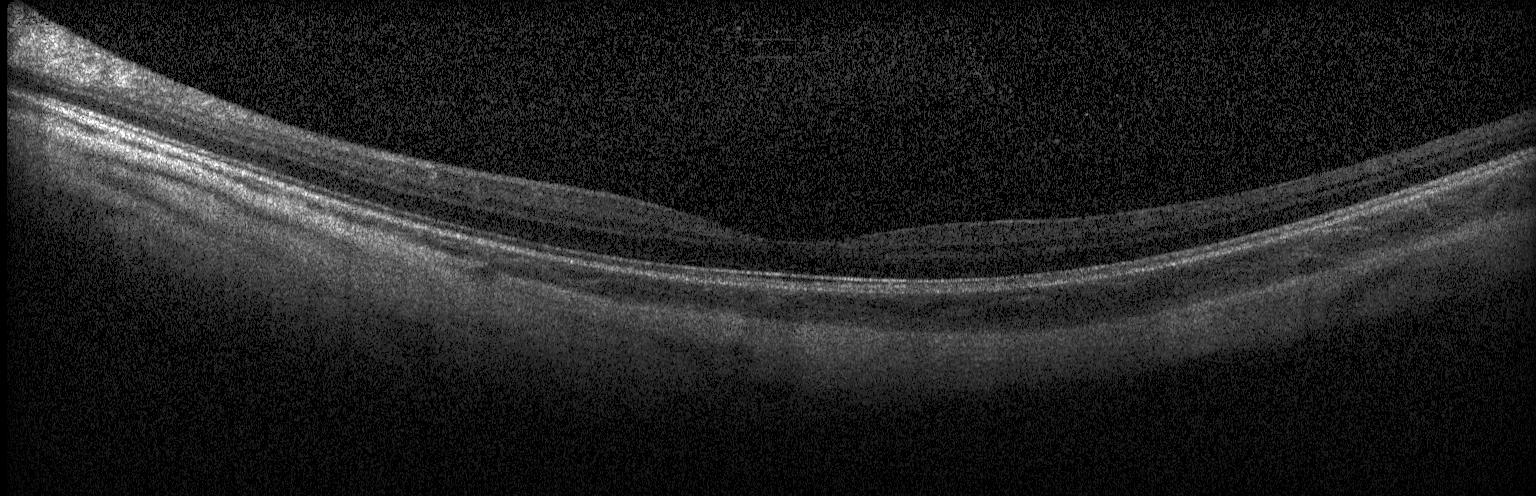

The scan shows no choroidal neovascularization, diabetic macular edema, or drusen.